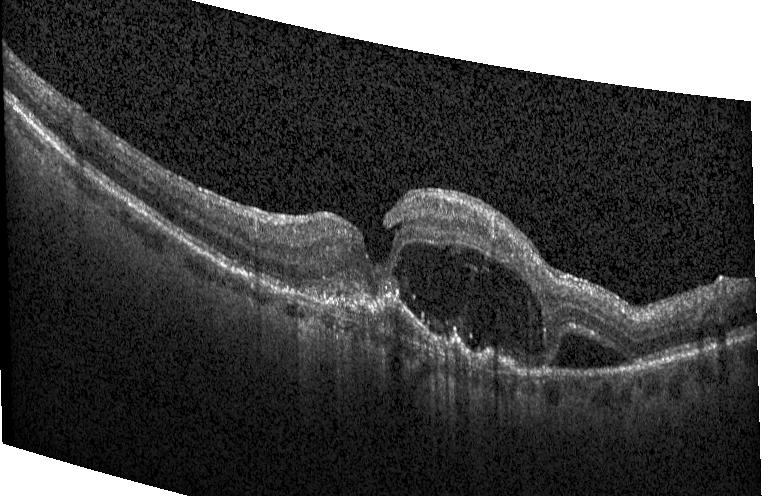

Diagnosis: a choroidal neovascular membrane.